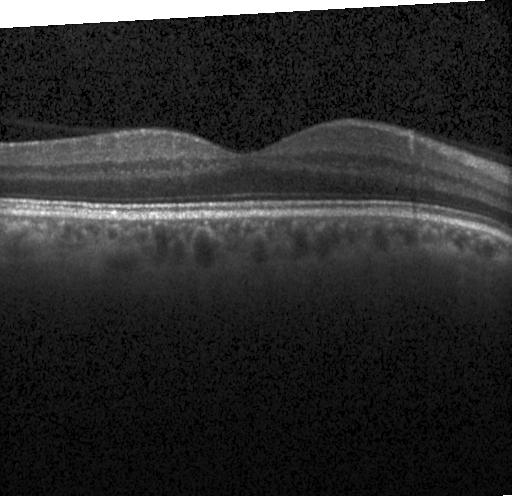 Through the macula. Spectral-domain OCT. OCT B-scan. Heidelberg Spectralis OCT system.
Assessment: no evidence of CNV, DME, or drusen.